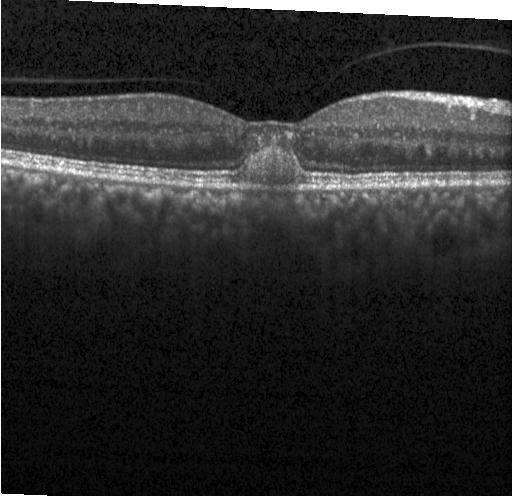 Instrument: Heidelberg Spectralis · retinal OCT B-scan — Assessment: a choroidal neovascular membrane.